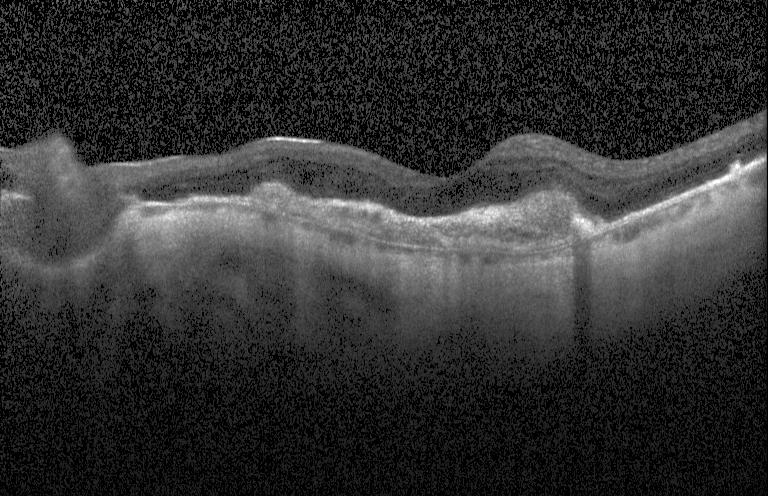

Acquired on a Heidelberg Spectralis, optical coherence tomography B-scan, macular scan. Assessment: choroidal neovascularization.